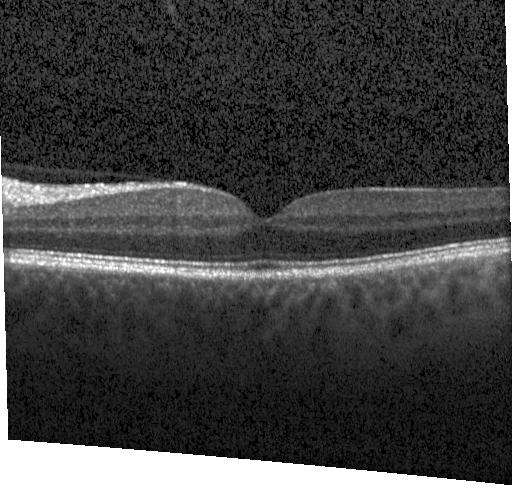 No choroidal neovascularization, diabetic macular edema, or drusen.